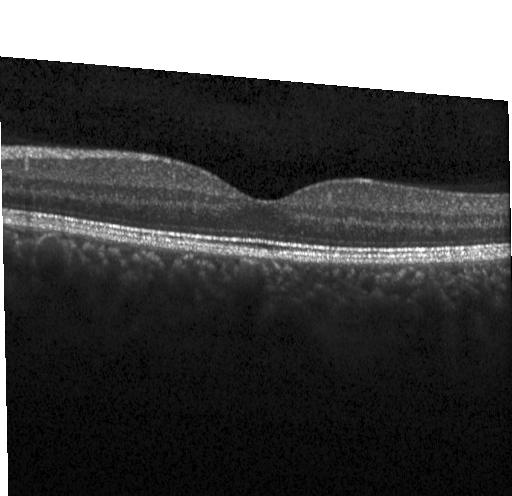 Finding: no choroidal neovascularization, diabetic macular edema, or drusen.